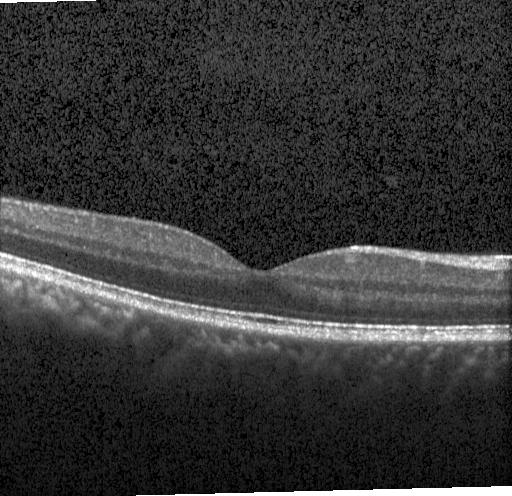
Retinal OCT cross-section. Spectral-domain optical coherence tomography
Diagnosis: neither choroidal neovascularization, diabetic macular edema, nor drusen.